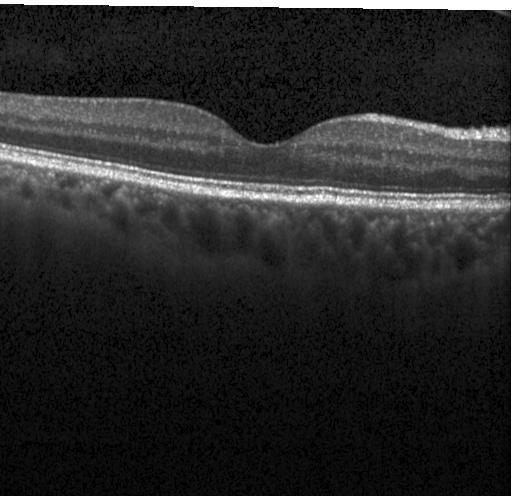

Impression: no evidence of choroidal neovascularization, diabetic macular edema, or drusen.